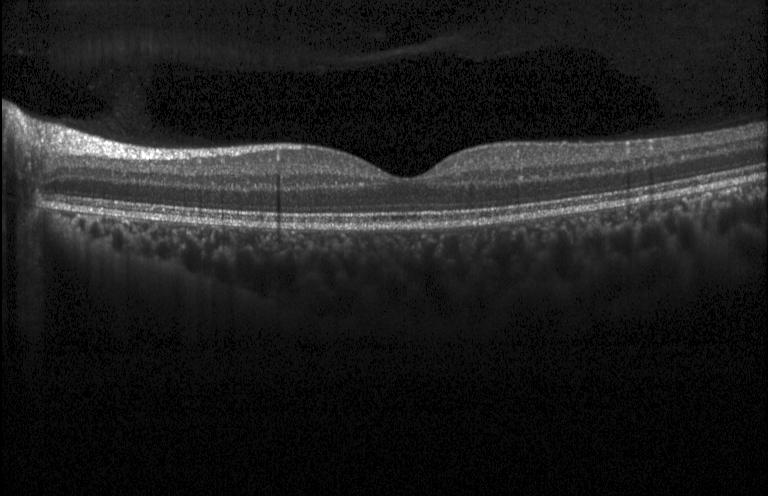 Impression: no CNV, no DME, and no drusen.